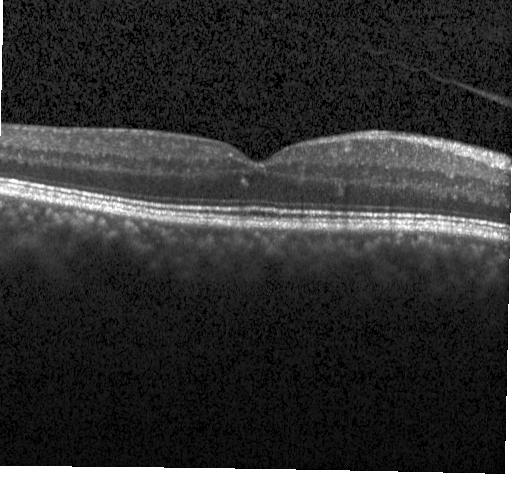
Heidelberg Spectralis OCT system · OCT line scan · SD-OCT. Diagnosis: no choroidal neovascularization, diabetic macular edema, or drusen.